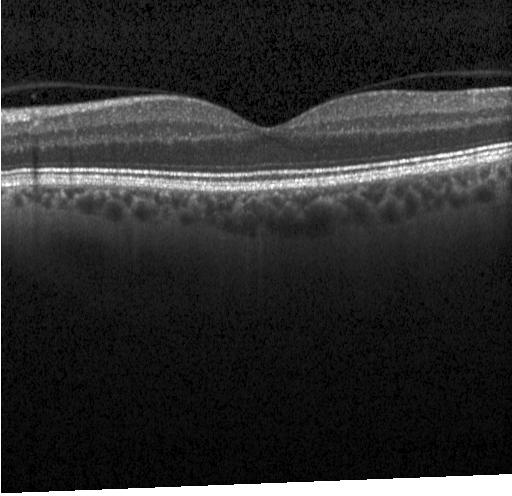 Diagnosis: no evidence of choroidal neovascularization, diabetic macular edema, or drusen.